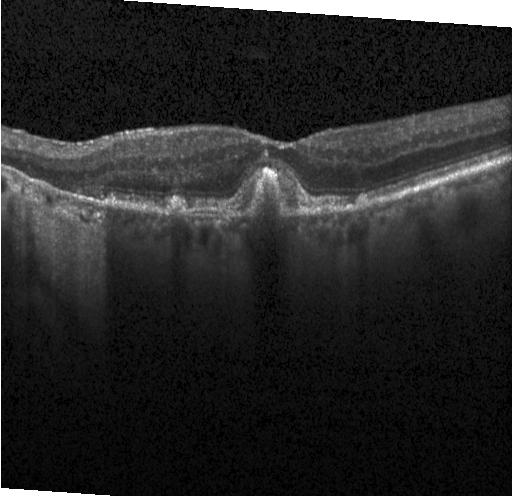
Retinal OCT B-scan; Heidelberg Spectralis; SD-OCT. Finding: a choroidal neovascular membrane.